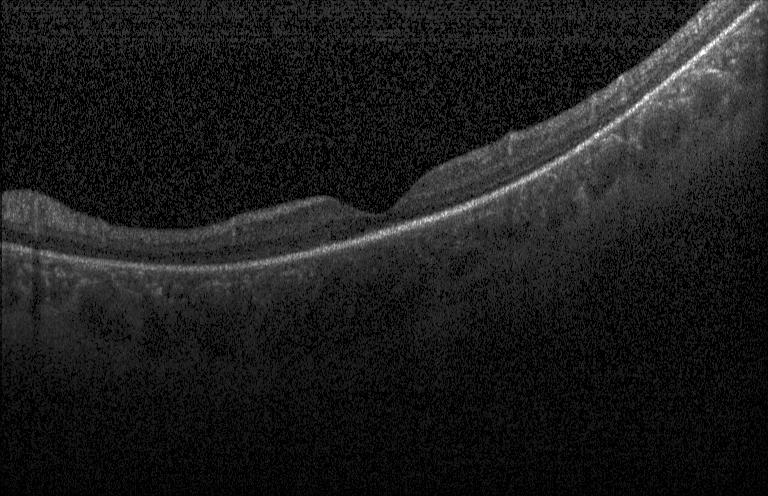
OCT scan showing neither CNV, DME, nor drusen.